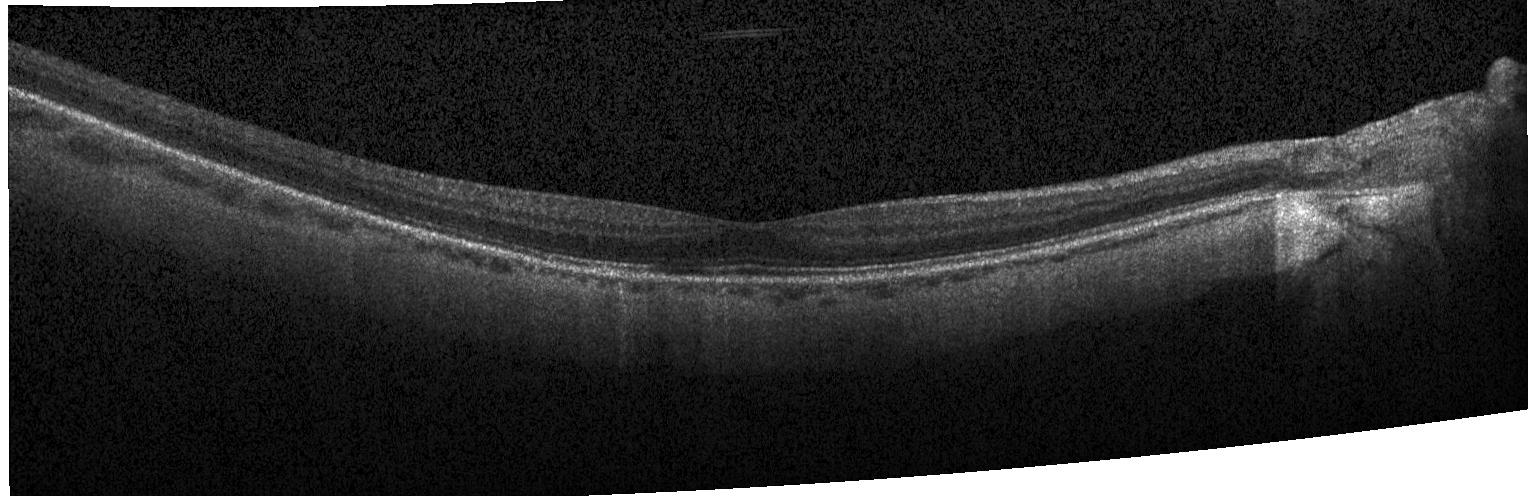

Optical coherence tomography scan. Impression: no evidence of choroidal neovascularization, diabetic macular edema, or drusen.